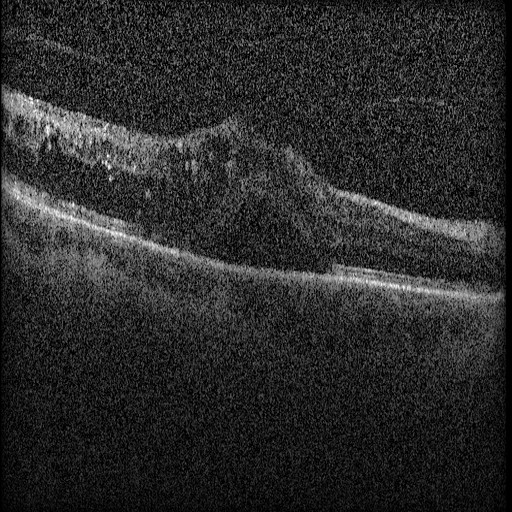
Impression: diabetic macular edema.